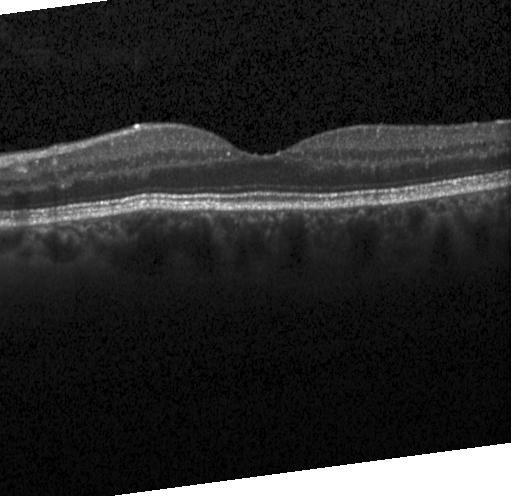
OCT B-scan. Macular scan. Spectral-domain optical coherence tomography — Diagnosis: neither CNV, DME, nor drusen.